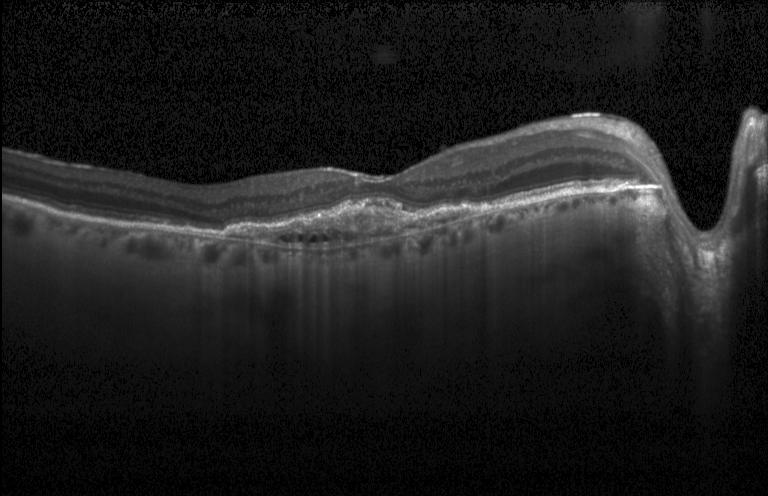
Retinal OCT cross-section showing a choroidal neovascular membrane.